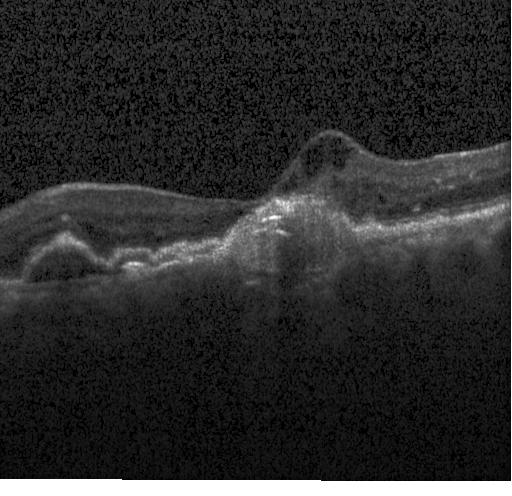
Macular OCT: choroidal neovascularization (CNV).